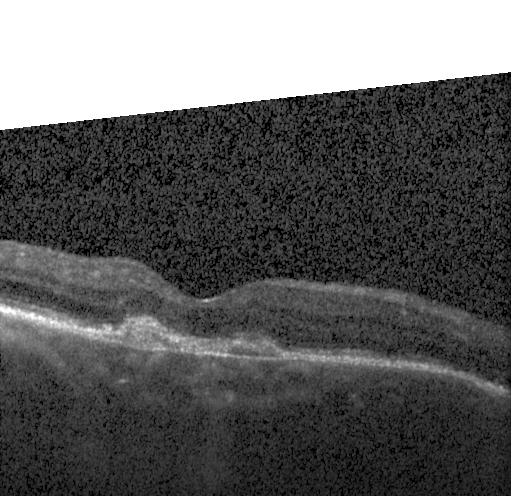
Retinal OCT B-scan. Through the macula — Macular OCT: a choroidal neovascular membrane.